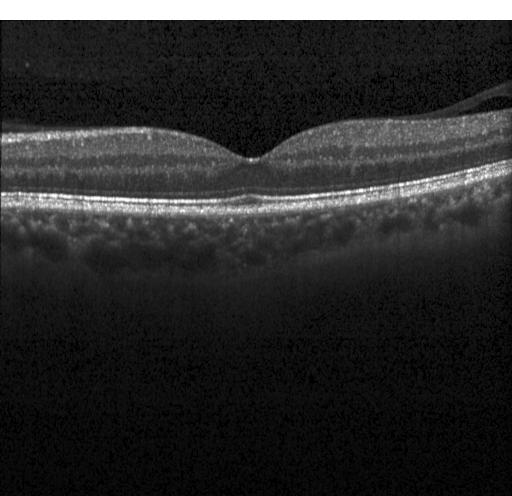 Retinal OCT B-scan — Diagnosis: no evidence of choroidal neovascularization, diabetic macular edema, or drusen.